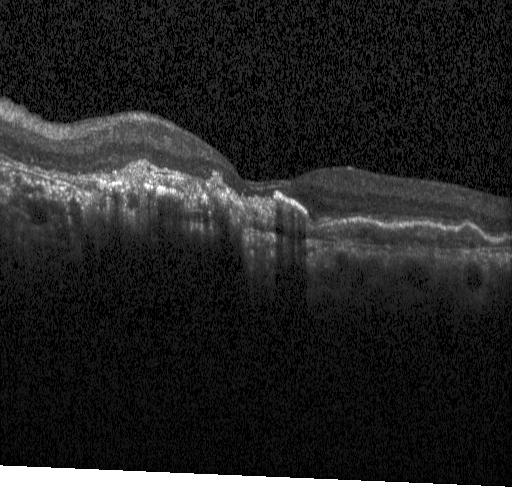

Retinal OCT B-scan.
Impression: a choroidal neovascular membrane.